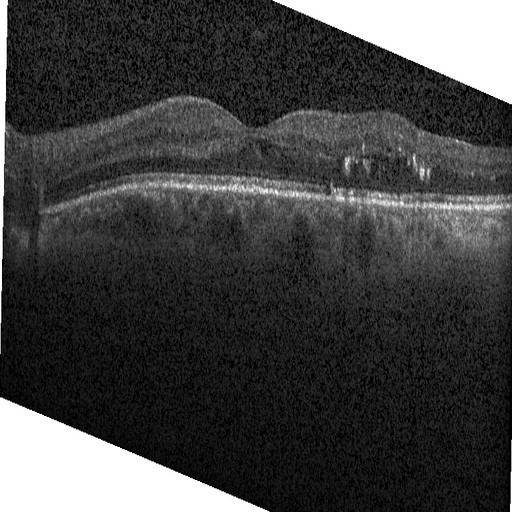 Retinal OCT cross-section — The scan shows DME.